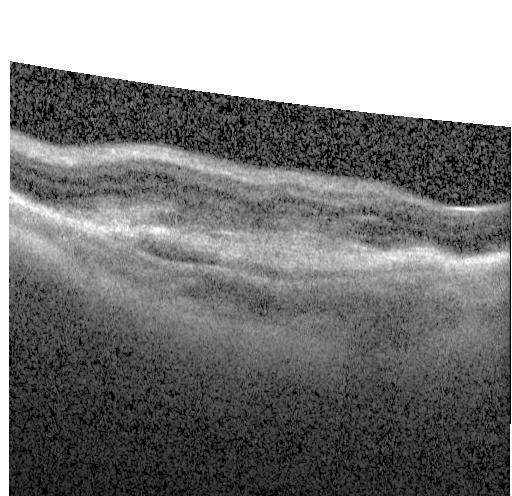

Centered on the fovea, instrument: Heidelberg Spectralis, retinal OCT B-scan, SD-OCT
Dx: CNV.